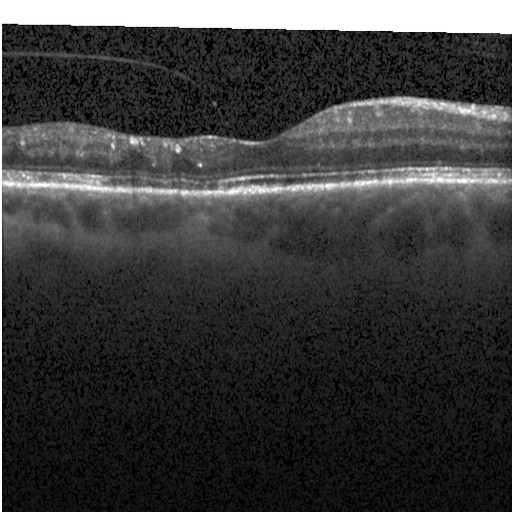 SD-OCT · optical coherence tomography scan — Finding: DME.